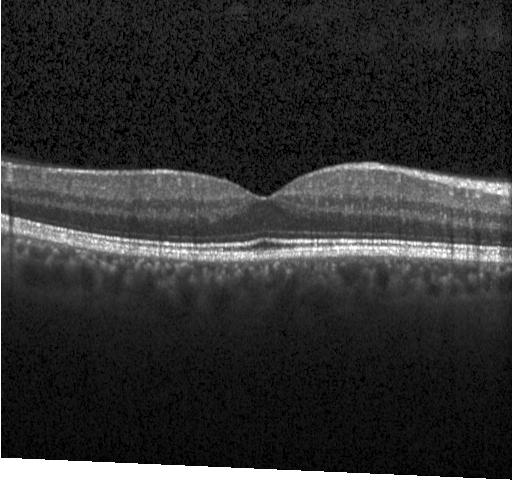

Macular OCT: no CNV, DME, or drusen.